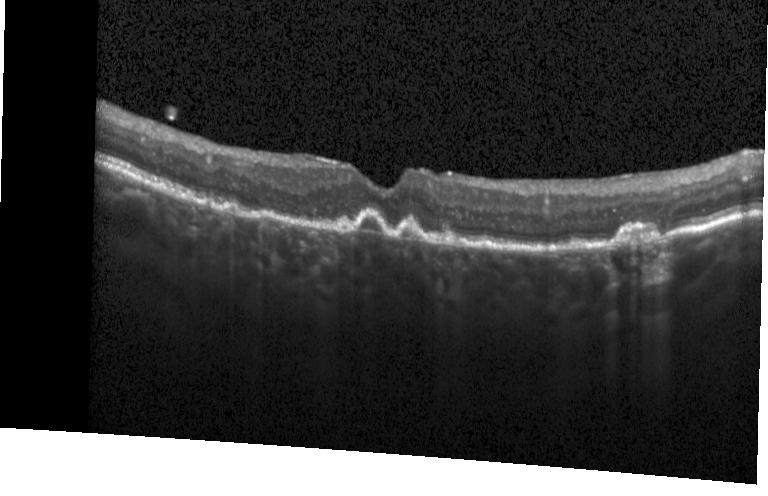 Fovea-centered. Retinal OCT B-scan. Spectral-domain optical coherence tomography. Instrument: Heidelberg Spectralis.
Dx: a choroidal neovascular membrane.